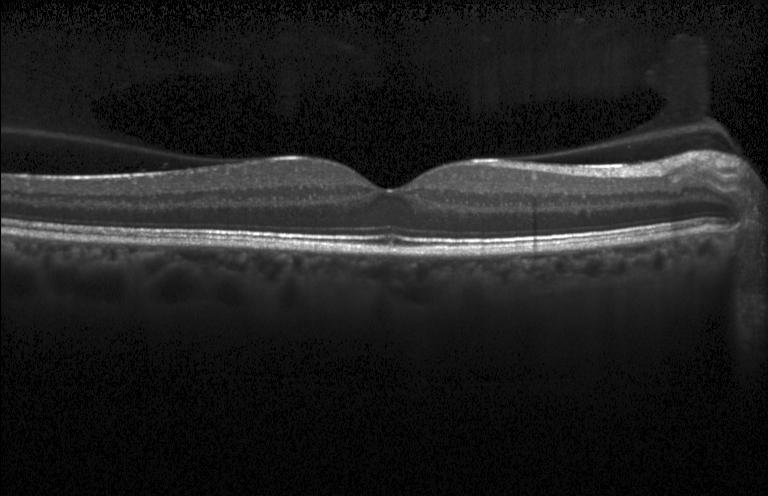
This B-scan demonstrates neither CNV, DME, nor drusen.